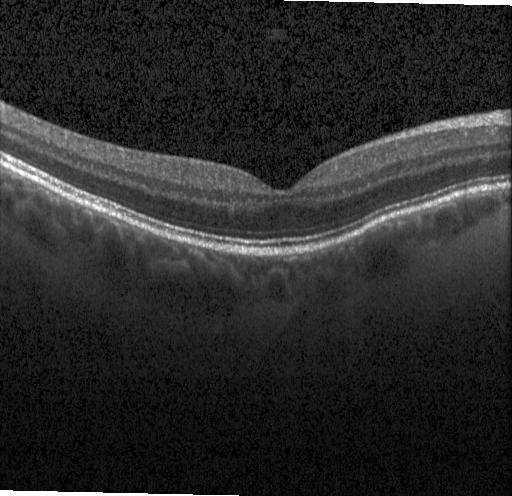

Through the macula; spectral-domain optical coherence tomography; OCT line scan.
Impression: no choroidal neovascularization, no diabetic macular edema, and no drusen.